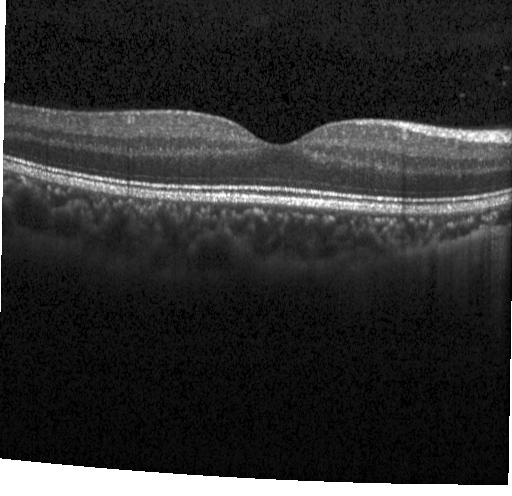
Retinal OCT cross-section; SD-OCT. This B-scan demonstrates no evidence of choroidal neovascularization, diabetic macular edema, or drusen.